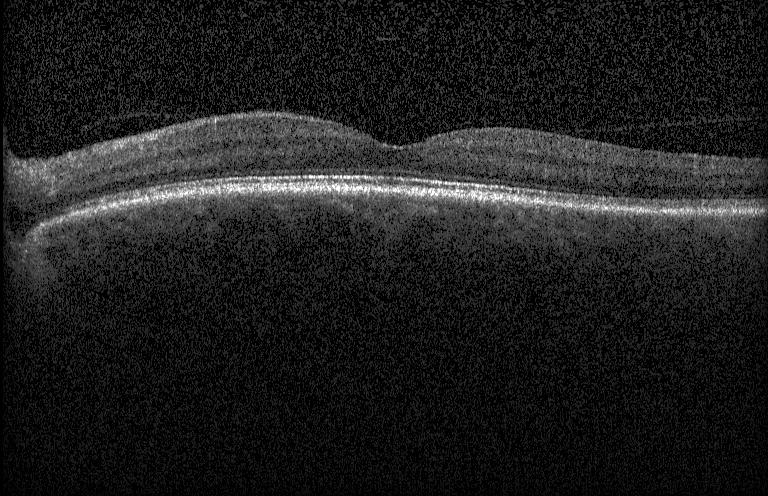
OCT B-scan. Diagnosis: no evidence of CNV, DME, or drusen.